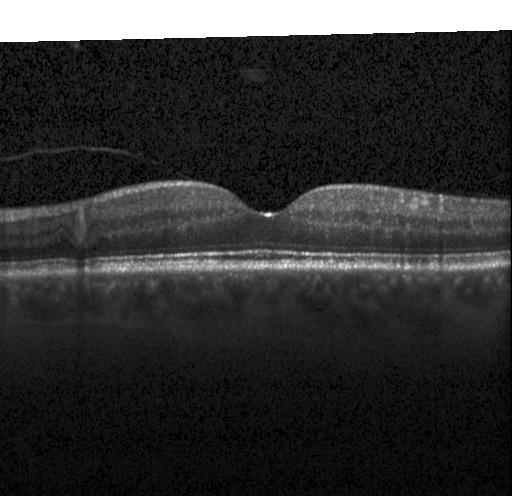
OCT line scan; SD-OCT
Finding: no CNV, no DME, and no drusen.